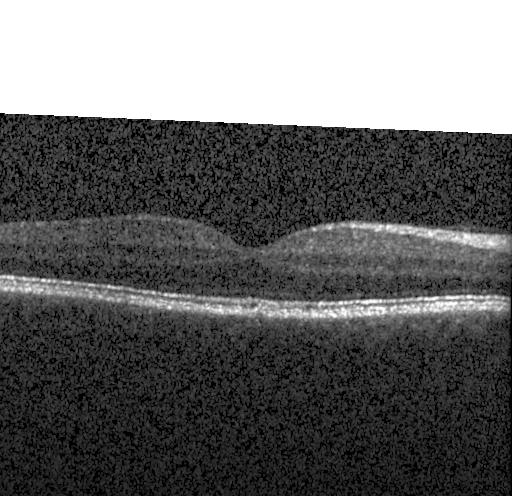
Optical coherence tomography scan.
Diagnosis: no choroidal neovascularization, no diabetic macular edema, and no drusen.